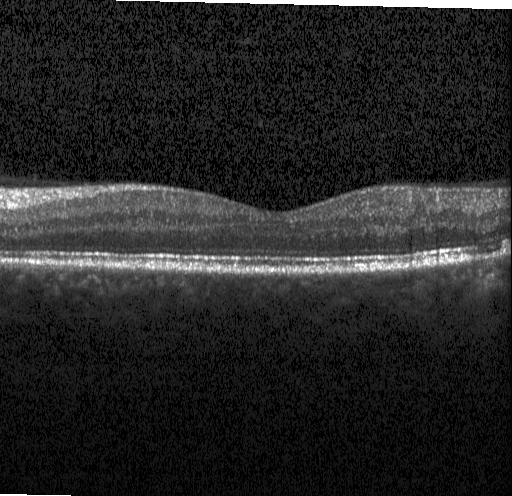

Retinal OCT B-scan, Heidelberg Spectralis, spectral-domain optical coherence tomography.
Impression: no CNV, DME, or drusen.